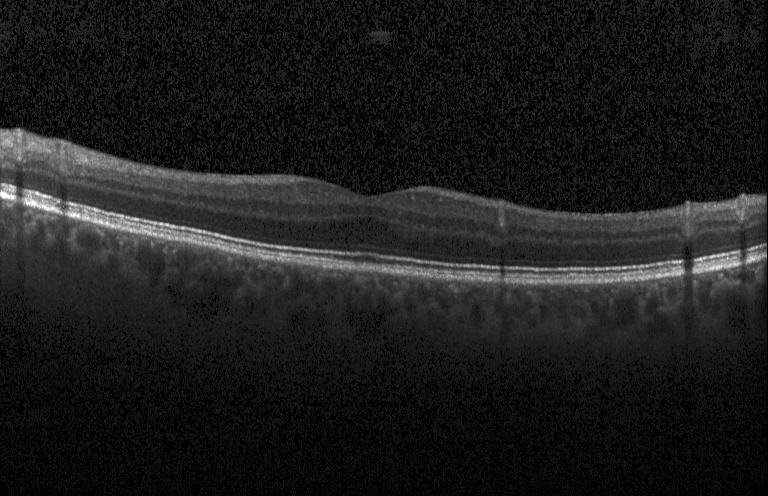 Retinal OCT cross-section.
Impression: no choroidal neovascularization, diabetic macular edema, or drusen.